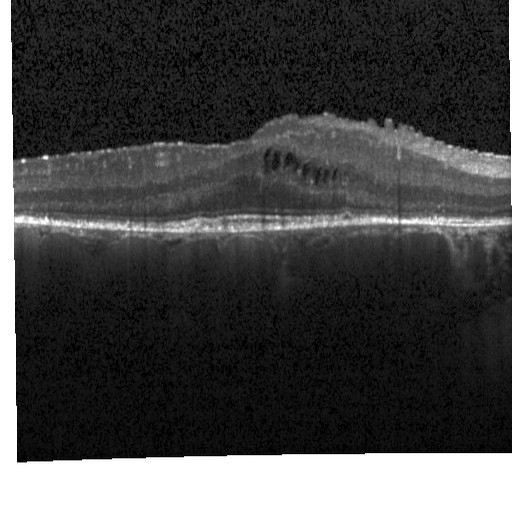 Retinal OCT B-scan, horizontal scan through the fovea, Heidelberg Spectralis. Diagnosis: diabetic macular edema.